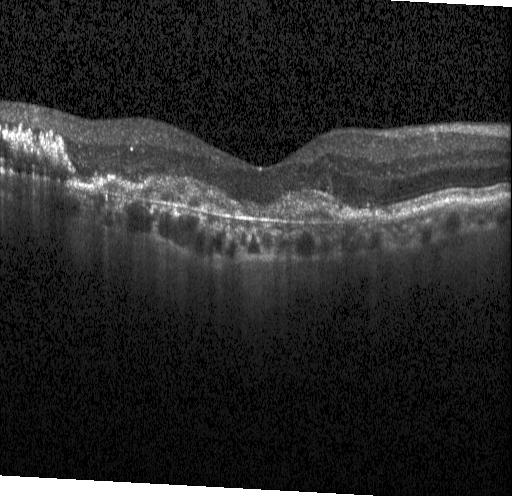 Optical coherence tomography B-scan, spectral-domain optical coherence tomography, Heidelberg Spectralis OCT system, through the macula.
Impression: a choroidal neovascular membrane.